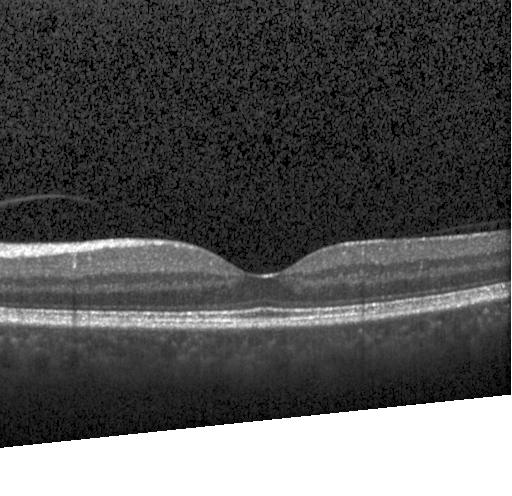 Assessment: no choroidal neovascularization, diabetic macular edema, or drusen.